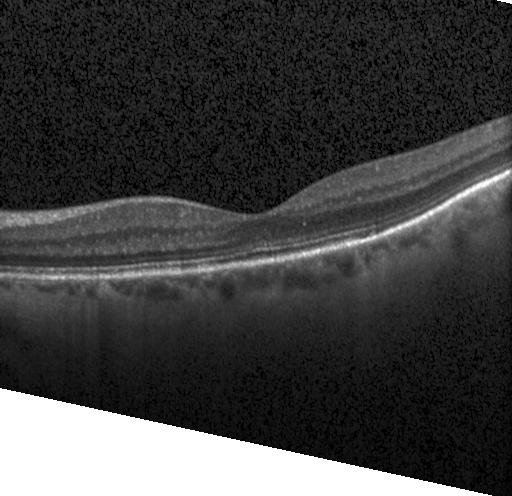
Spectral-domain OCT B-scan: neither CNV, DME, nor drusen.